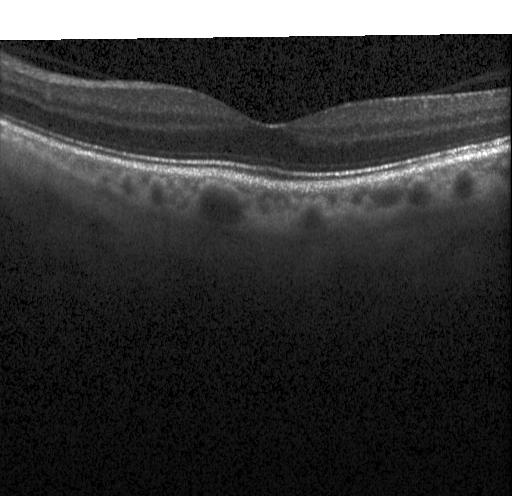

OCT B-scan. Horizontal scan through the fovea.
Diagnosis: no CNV, DME, or drusen.